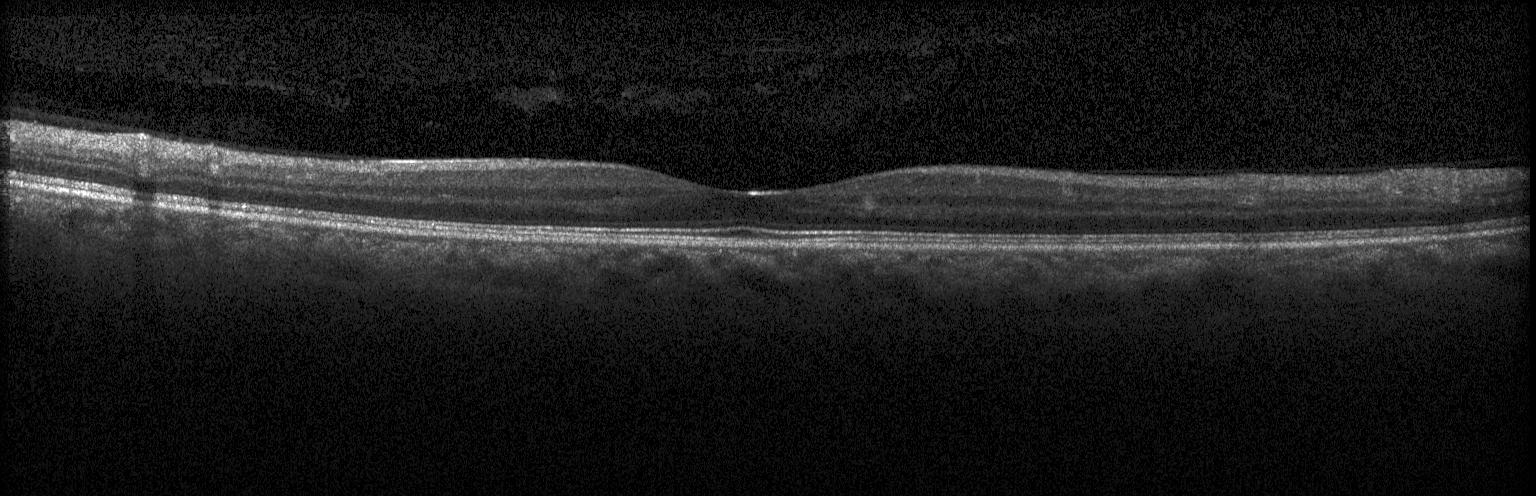 Macular scan, OCT line scan, spectral-domain OCT, instrument: Heidelberg Spectralis.
Diagnosis: no evidence of choroidal neovascularization, diabetic macular edema, or drusen.